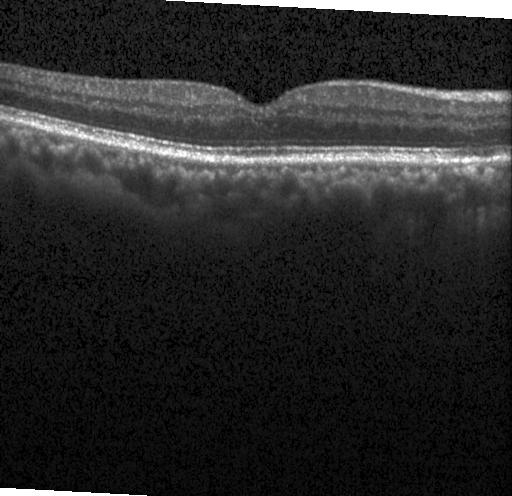
This B-scan demonstrates neither choroidal neovascularization, diabetic macular edema, nor drusen.